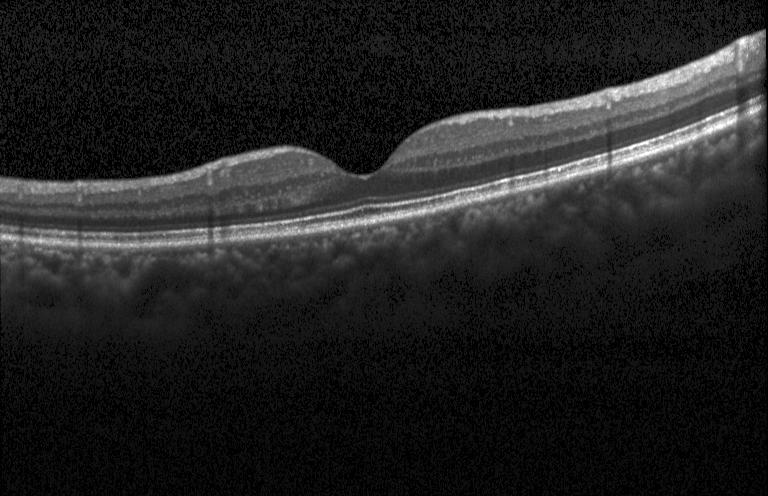
Optical coherence tomography scan · fovea-centered · SD-OCT. Finding: no choroidal neovascularization, no diabetic macular edema, and no drusen.